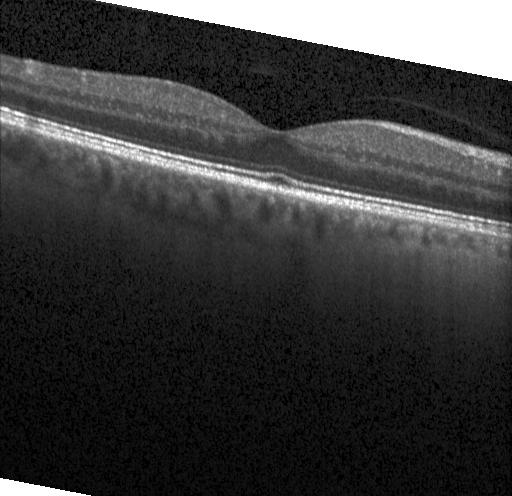 Optical coherence tomography B-scan — Assessment: no evidence of choroidal neovascularization, diabetic macular edema, or drusen.